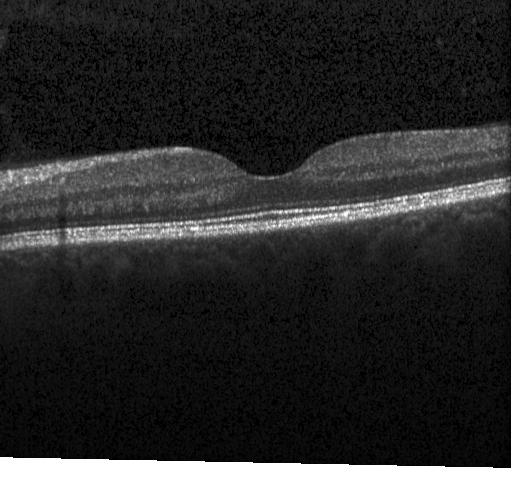
Retinal OCT B-scan, fovea-centered, Heidelberg Spectralis, spectral-domain OCT.
Neither choroidal neovascularization, diabetic macular edema, nor drusen.